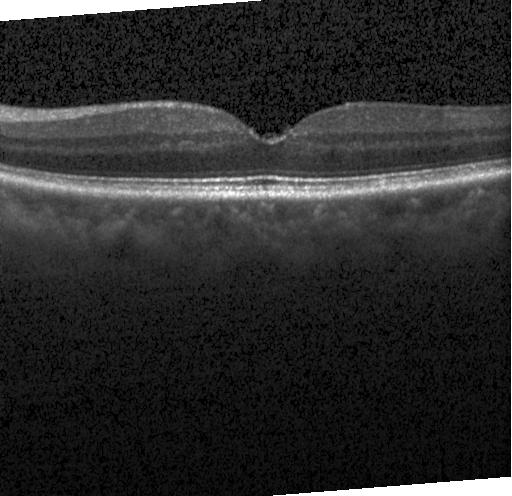

OCT line scan. Heidelberg Spectralis OCT system. Spectral-domain optical coherence tomography. Fovea-centered. Impression: neither choroidal neovascularization, diabetic macular edema, nor drusen.